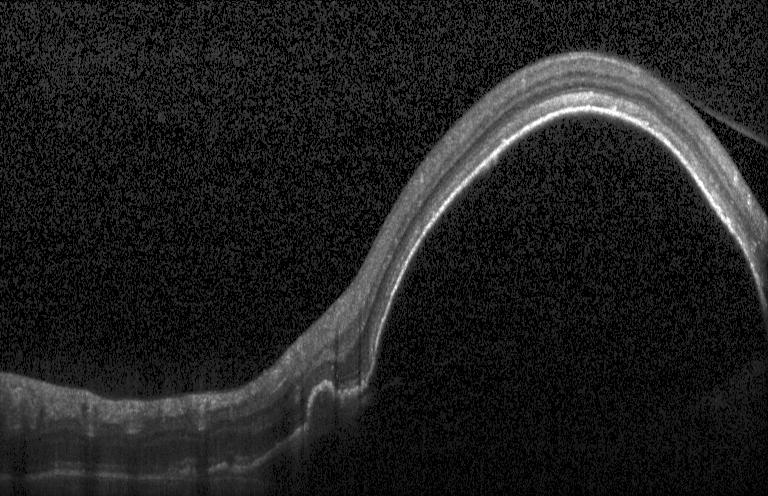 Optical coherence tomography scan — This B-scan demonstrates choroidal neovascularization (CNV).